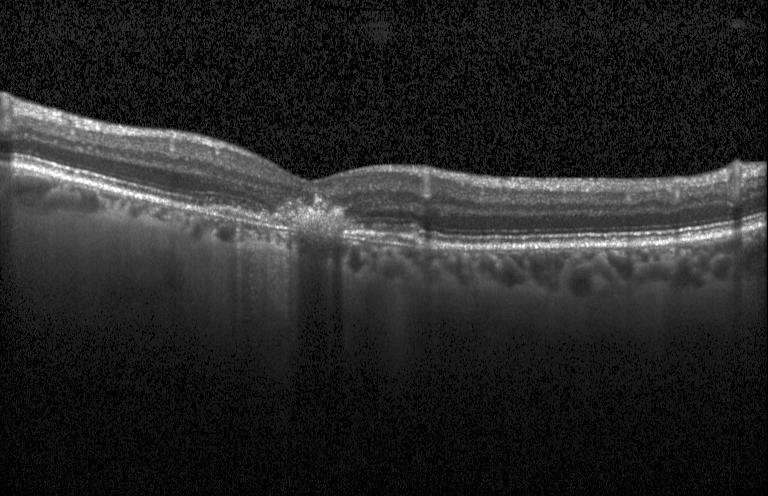 Instrument: Heidelberg Spectralis. Retinal OCT B-scan. Centered on the fovea — Impression: choroidal neovascularization (CNV).